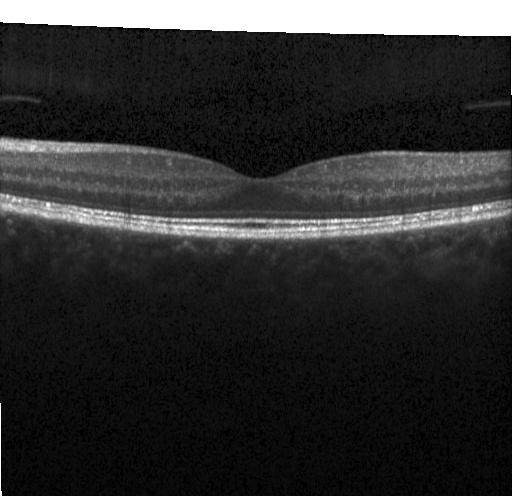

Dx: no CNV, no DME, and no drusen.